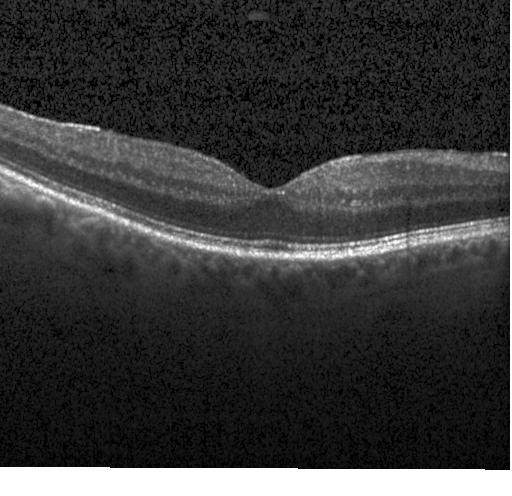

OCT B-scan, spectral-domain OCT, fovea-centered. Impression: no choroidal neovascularization, diabetic macular edema, or drusen.